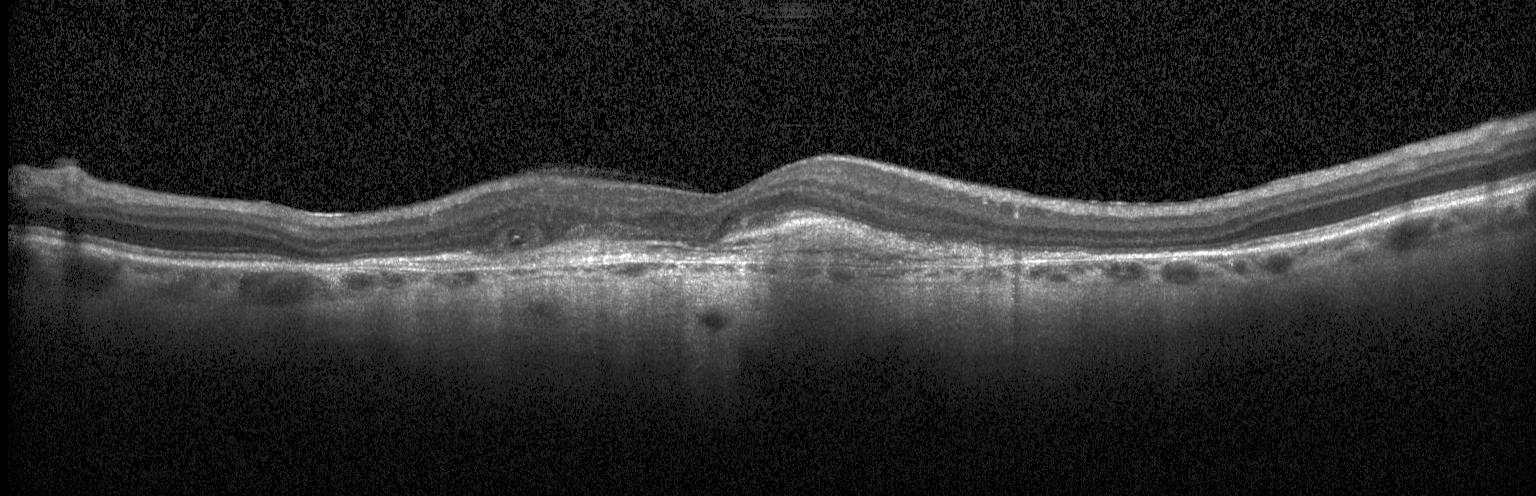
Optical coherence tomography scan · spectral-domain optical coherence tomography · horizontal scan through the fovea · Heidelberg Spectralis OCT system
The scan shows a choroidal neovascular membrane.